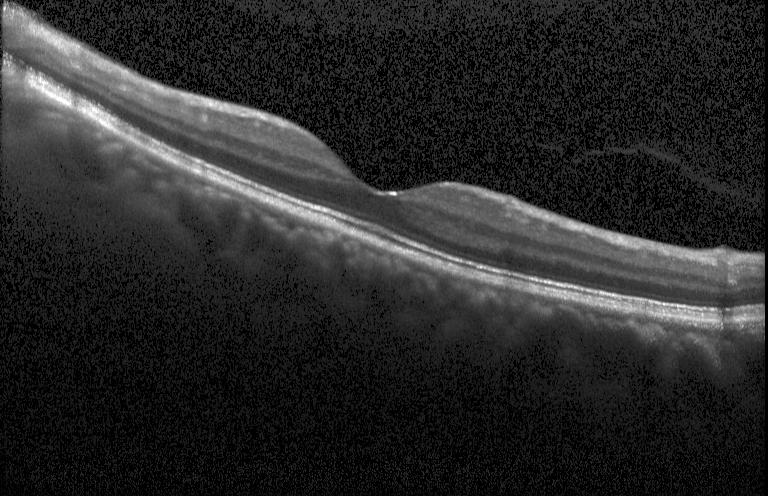 Heidelberg Spectralis; optical coherence tomography B-scan; centered on the fovea; SD-OCT
Impression: no evidence of choroidal neovascularization, diabetic macular edema, or drusen.